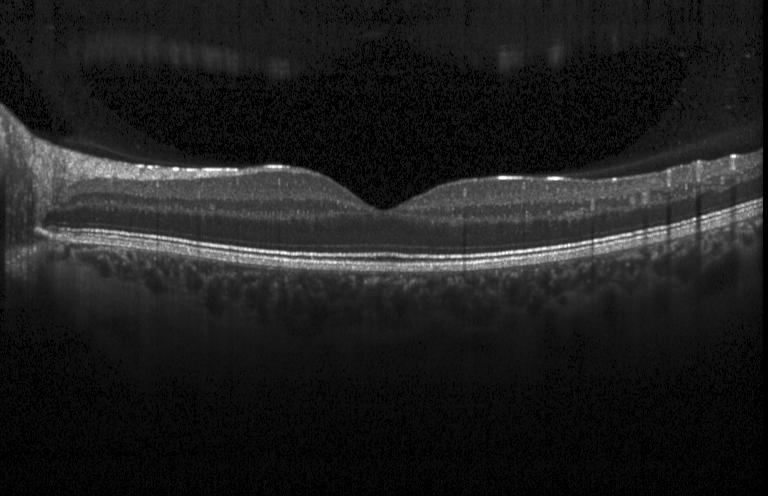 Macular scan. Spectral-domain OCT. Heidelberg Spectralis. Retinal OCT cross-section. Dx: neither choroidal neovascularization, diabetic macular edema, nor drusen.